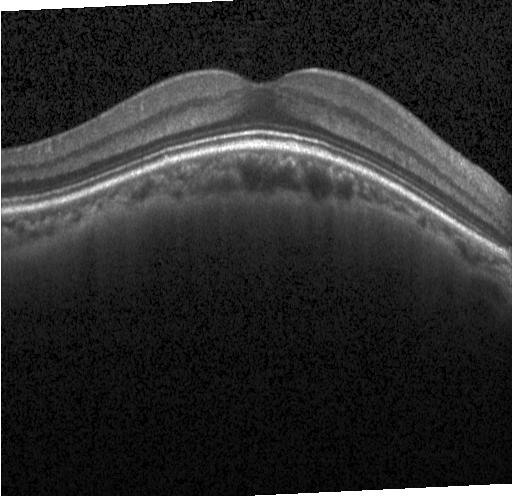

Diagnosis: no choroidal neovascularization, diabetic macular edema, or drusen.